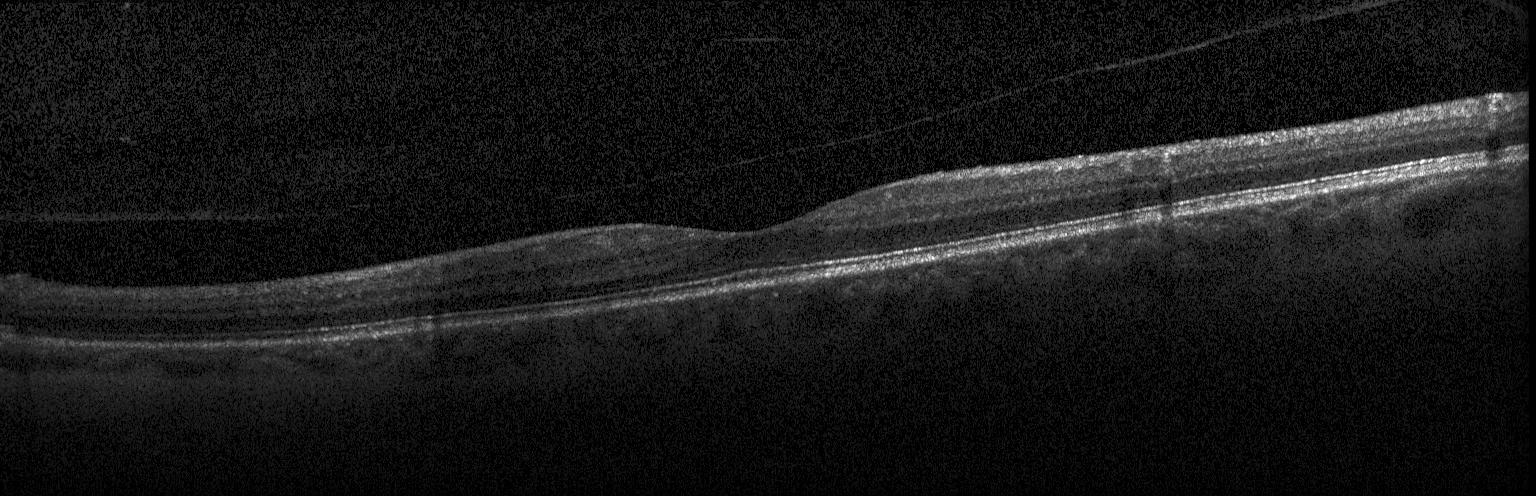

Retinal OCT cross-section showing neither choroidal neovascularization, diabetic macular edema, nor drusen.